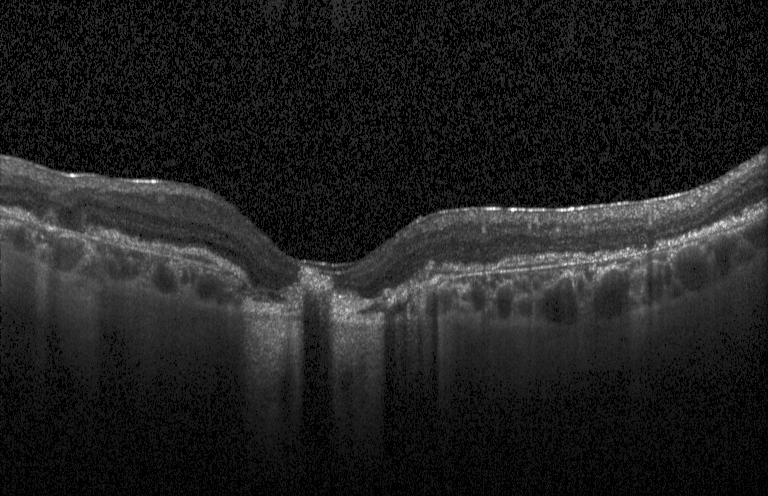
Diagnosis: choroidal neovascularization.